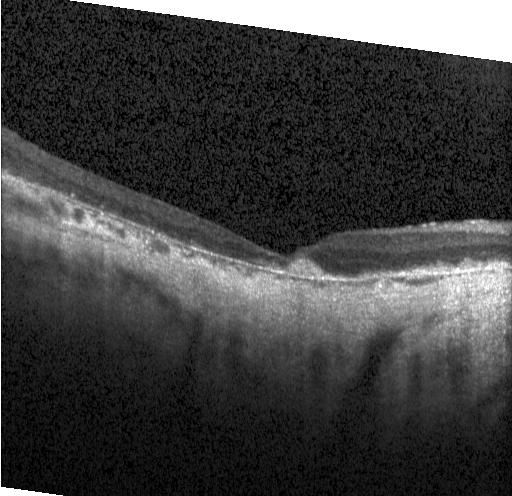
Spectral-domain OCT. Heidelberg Spectralis OCT system. Retinal OCT cross-section
Dx: choroidal neovascularization.